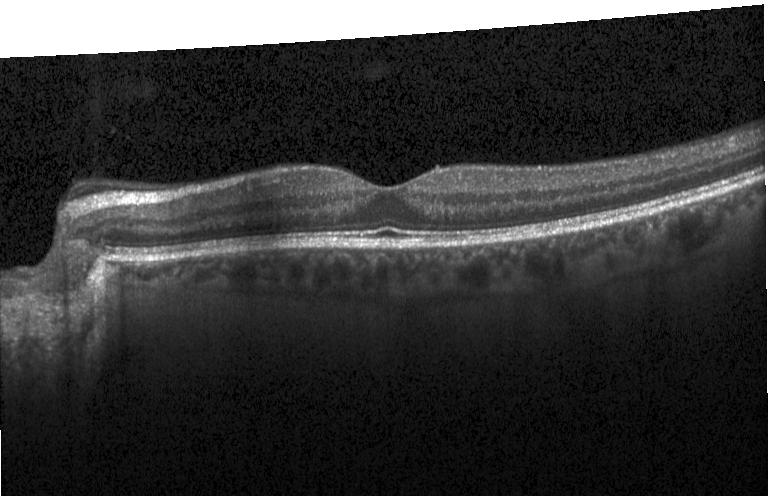

Heidelberg Spectralis · OCT B-scan — Diagnosis: neither choroidal neovascularization, diabetic macular edema, nor drusen.